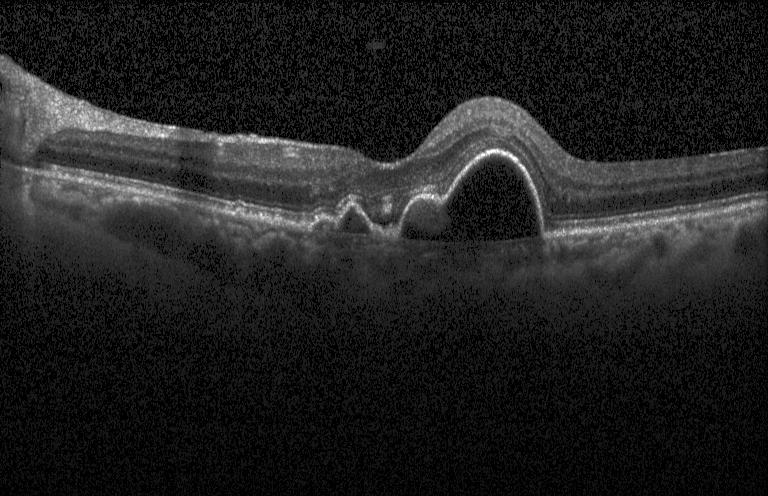 Optical coherence tomography B-scan · spectral-domain OCT. The scan shows choroidal neovascularization.